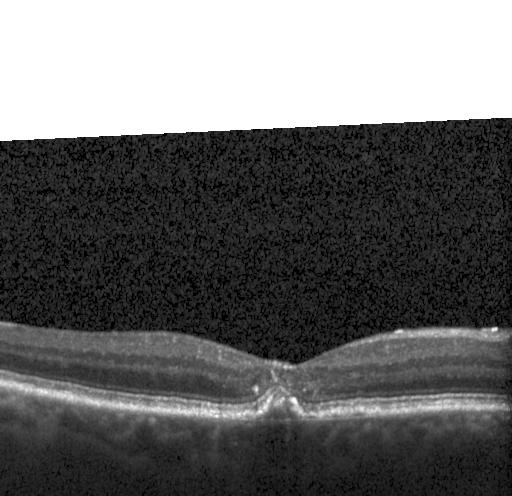

Heidelberg Spectralis OCT system. Spectral-domain optical coherence tomography. Macular scan. Optical coherence tomography scan — Finding: multiple drusen.